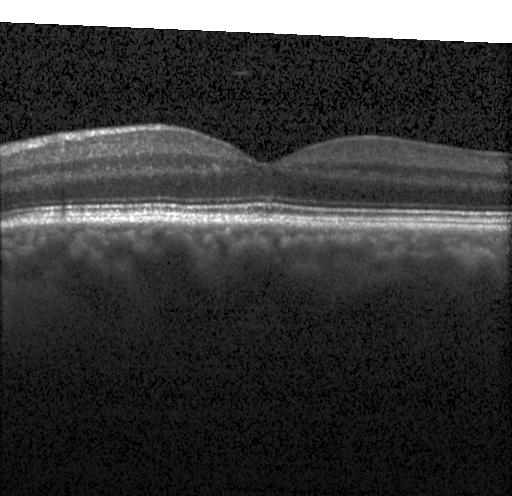
Retinal OCT cross-section; macular scan; acquired on a Heidelberg Spectralis. Impression: no CNV, DME, or drusen.